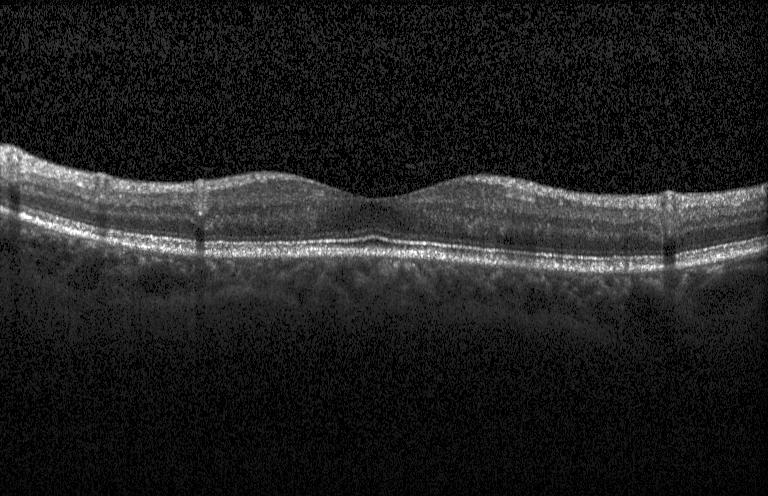
SD-OCT · Heidelberg Spectralis · OCT line scan.
Impression: no choroidal neovascularization, no diabetic macular edema, and no drusen.